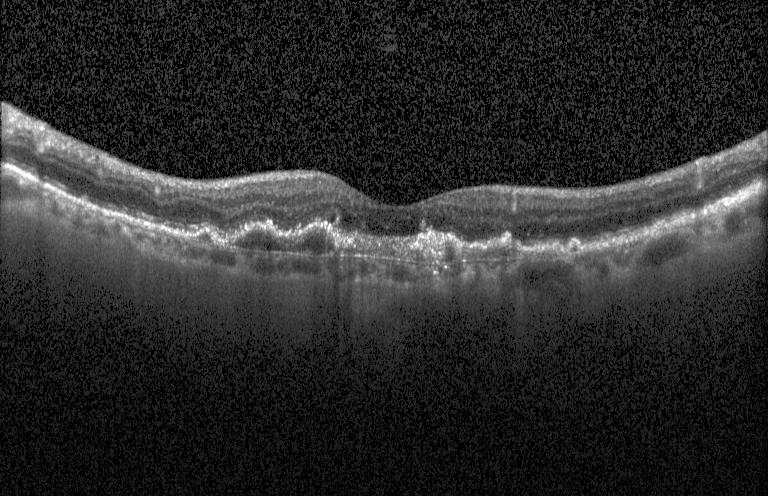 Impression: a choroidal neovascular membrane.